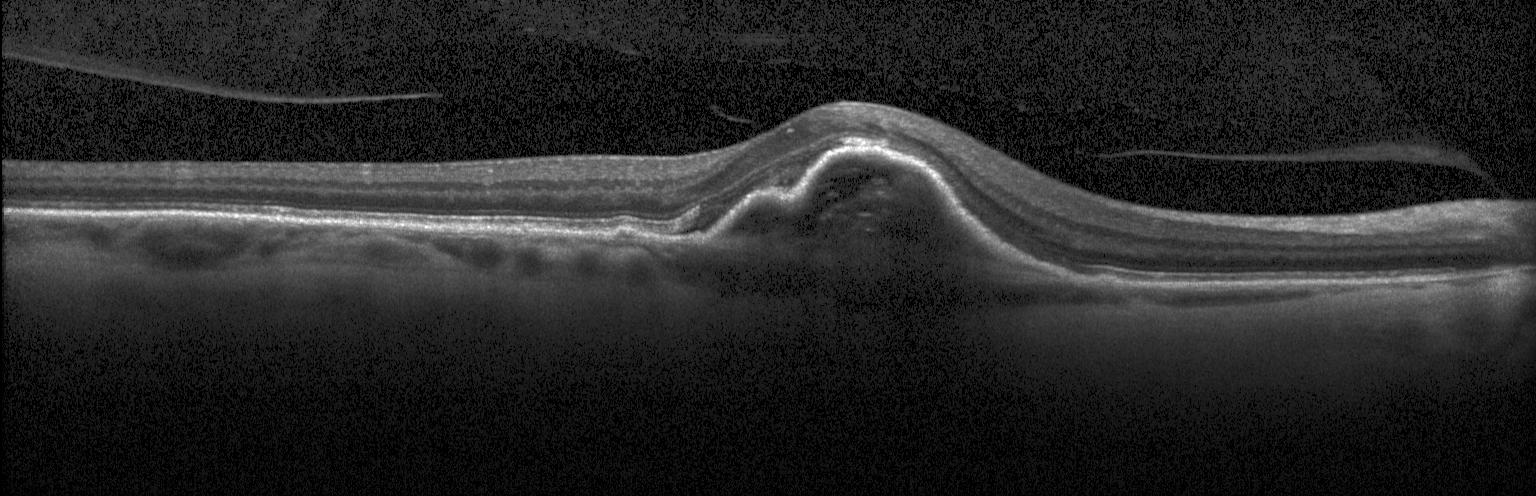

Acquired on a Heidelberg Spectralis · fovea-centered · retinal OCT B-scan.
Macular OCT: a choroidal neovascular membrane.